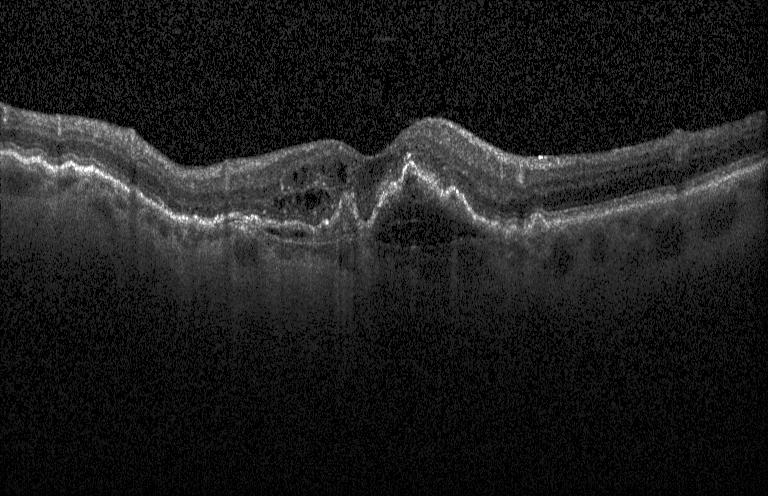 Optical coherence tomography scan. Dx: choroidal neovascularization.